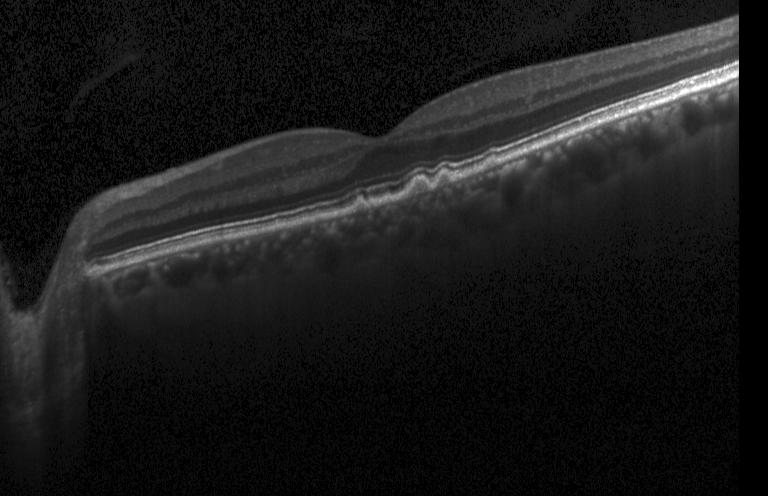
Horizontal scan through the fovea · retinal OCT cross-section · Heidelberg Spectralis OCT system · spectral-domain optical coherence tomography
Sub-RPE drusenoid deposits.